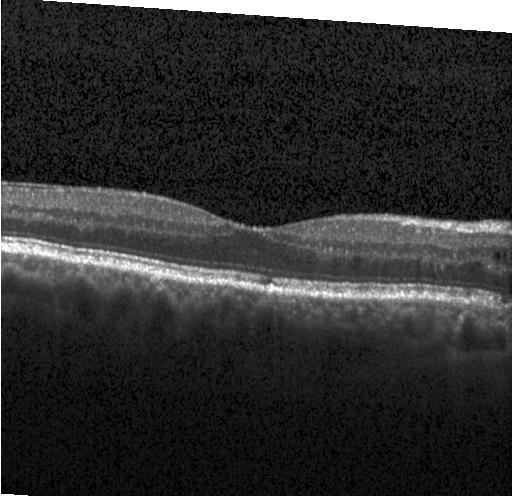 Retinal OCT cross-section showing diabetic macular edema.